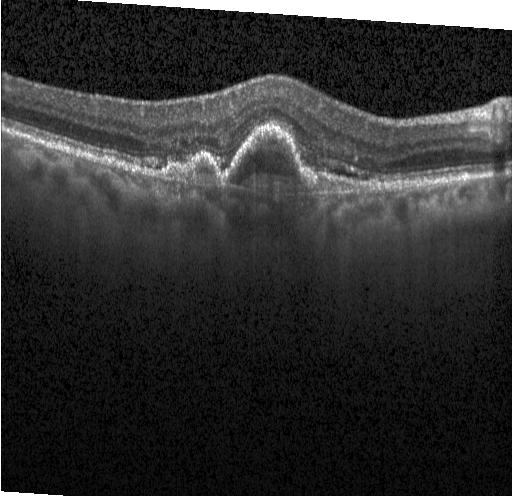 Heidelberg Spectralis · through the macula · spectral-domain OCT · optical coherence tomography B-scan — Assessment: choroidal neovascularization.